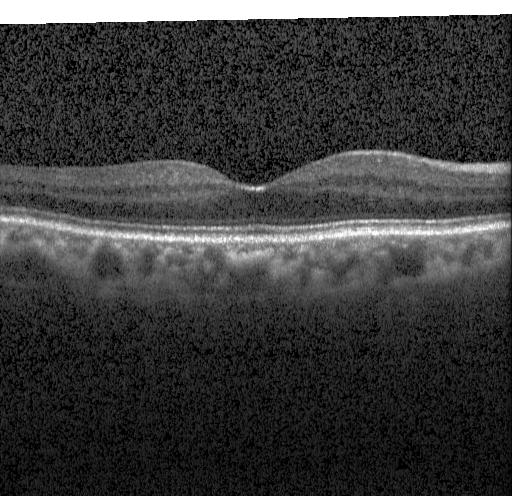
Diagnosis: no choroidal neovascularization, diabetic macular edema, or drusen.